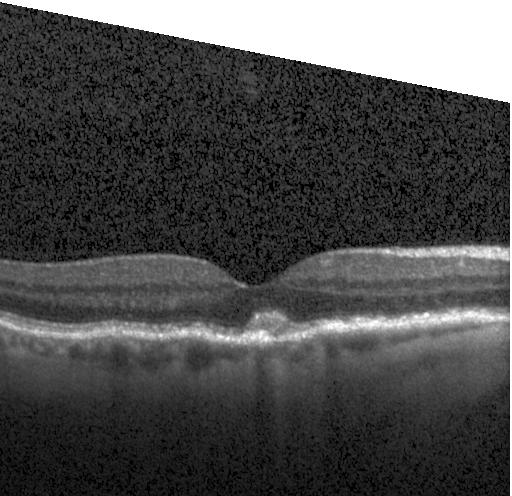
OCT line scan
Assessment: drusen.